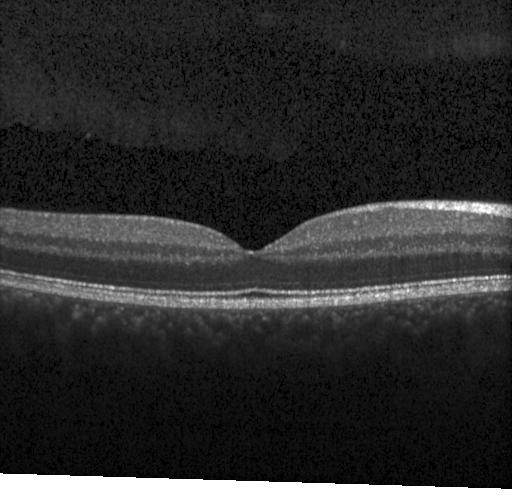
Instrument: Heidelberg Spectralis, OCT B-scan, centered on the fovea
Impression: no choroidal neovascularization, diabetic macular edema, or drusen.